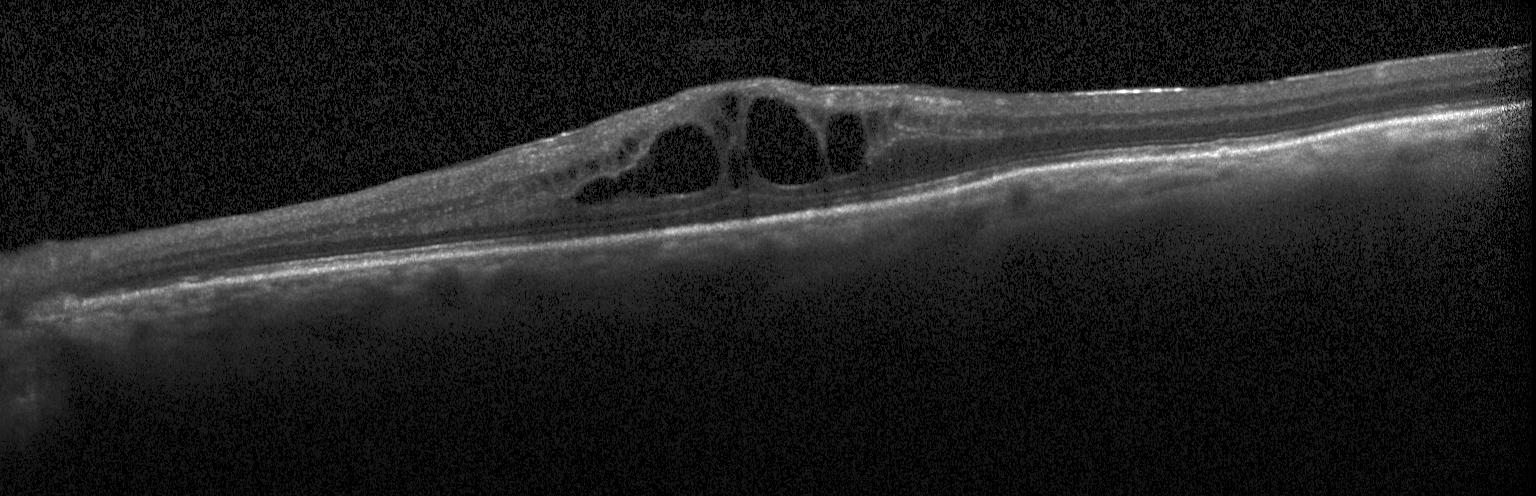

Diagnosis: diabetic macular edema.